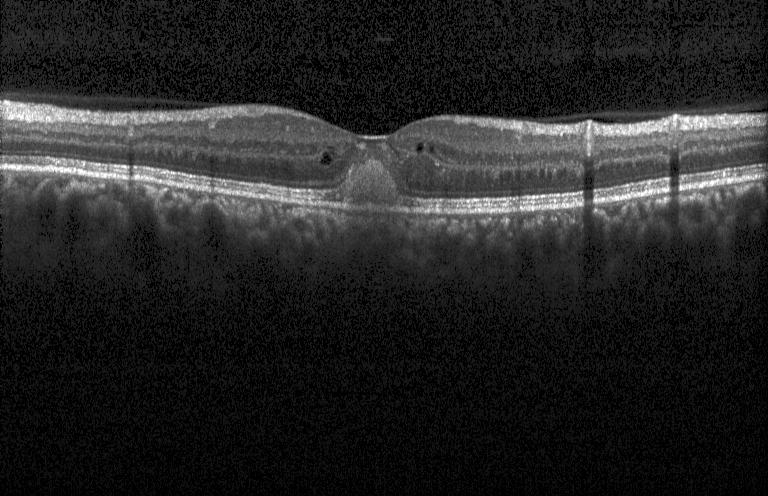 Optical coherence tomography B-scan.
Assessment: CNV.